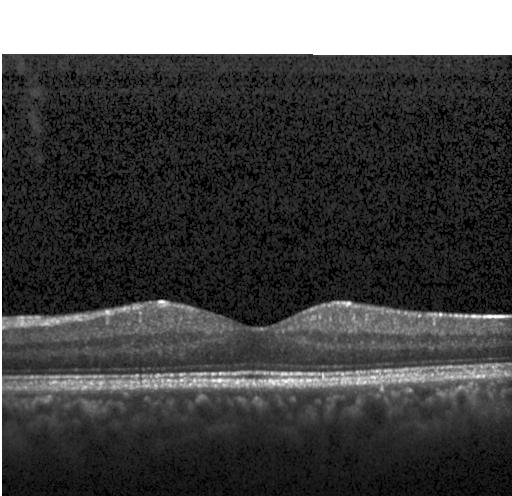

Dx: no CNV, DME, or drusen.